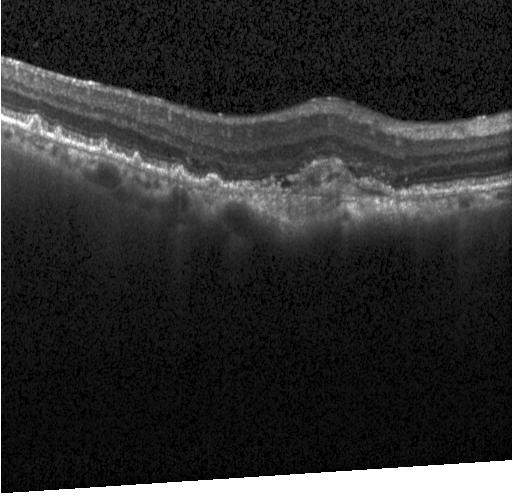
Optical coherence tomography B-scan.
Assessment: choroidal neovascularization.